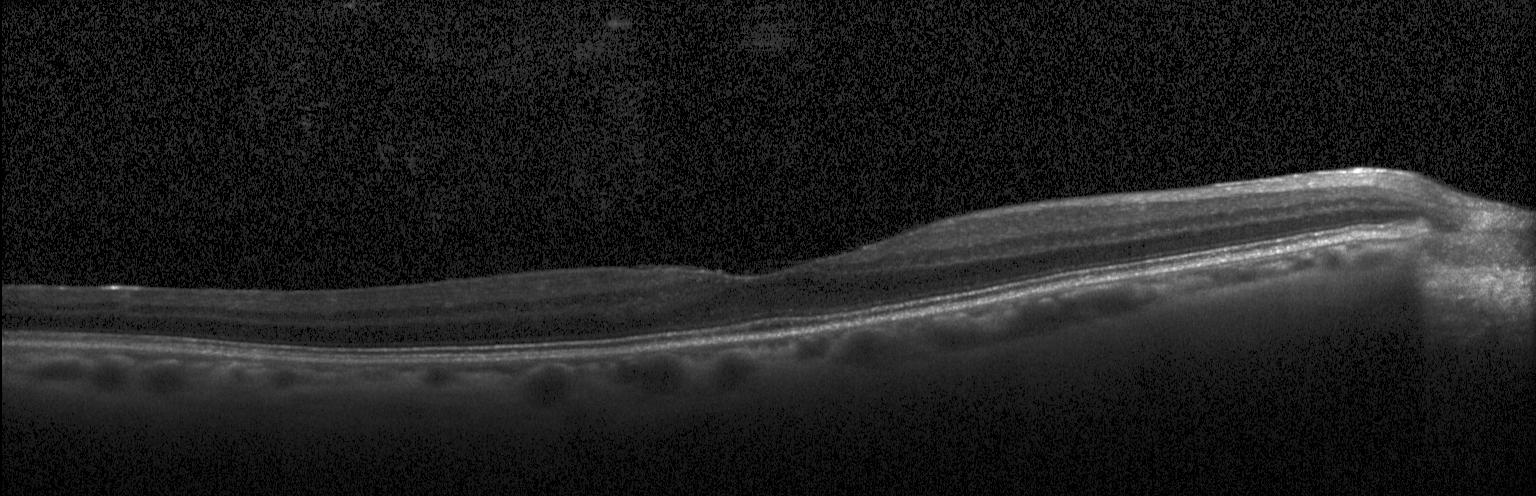

OCT finding: neither choroidal neovascularization, diabetic macular edema, nor drusen.